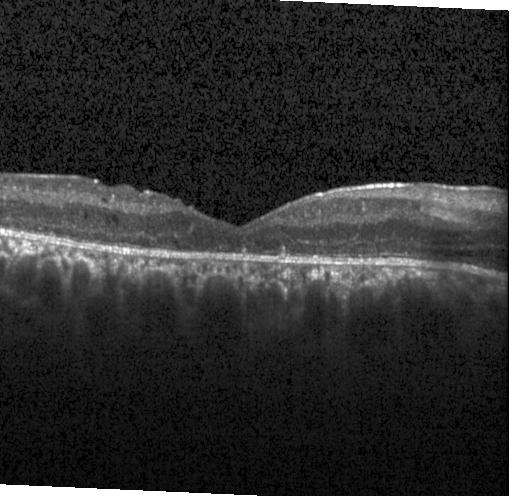
Impression: diabetic macular edema.